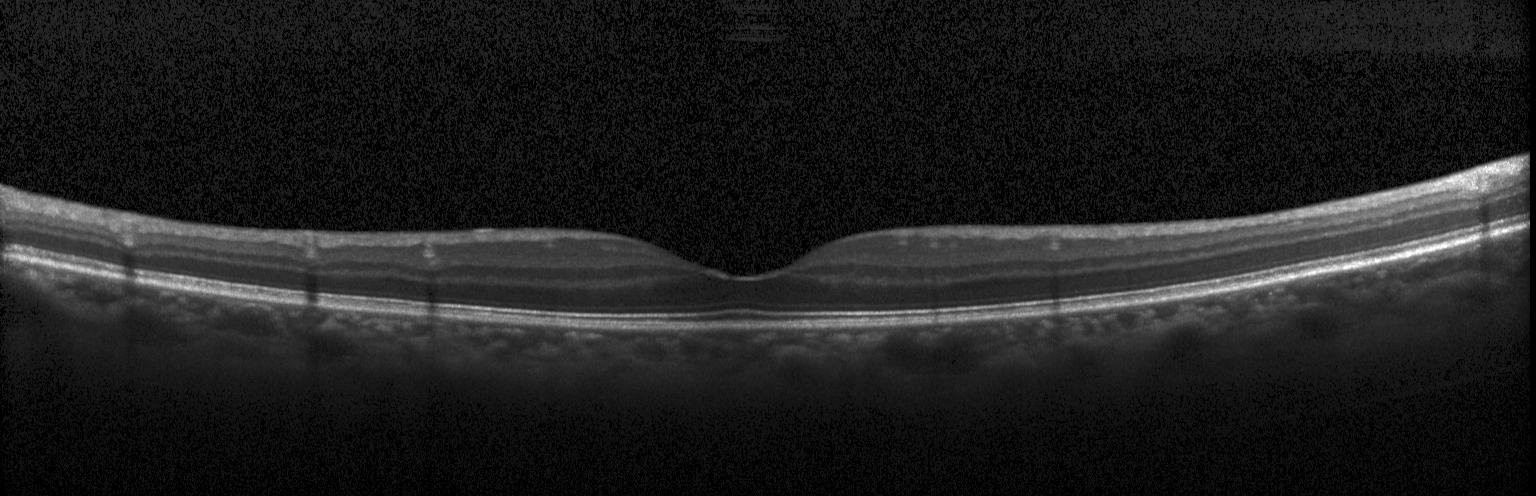
Finding: neither CNV, DME, nor drusen.